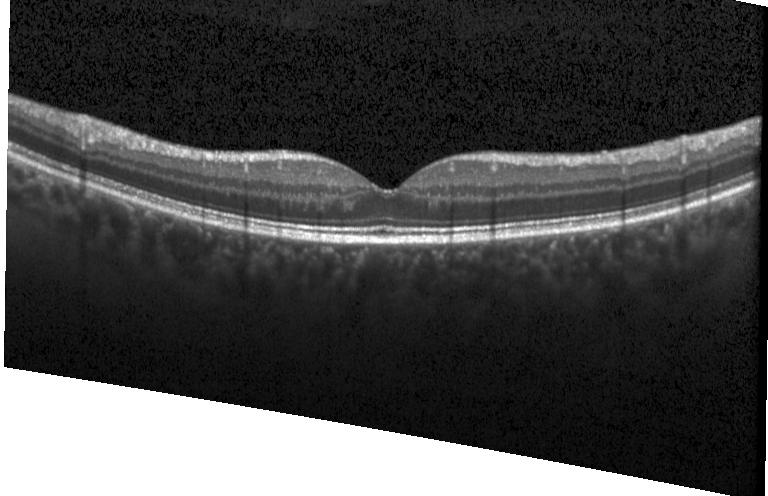
Retinal OCT cross-section, acquired on a Heidelberg Spectralis, through the macula — No choroidal neovascularization, no diabetic macular edema, and no drusen.